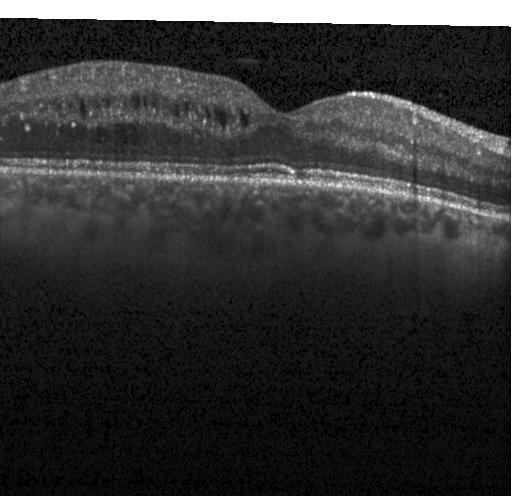 Optical coherence tomography B-scan. Spectral-domain OCT — Assessment: diabetic macular edema (DME).